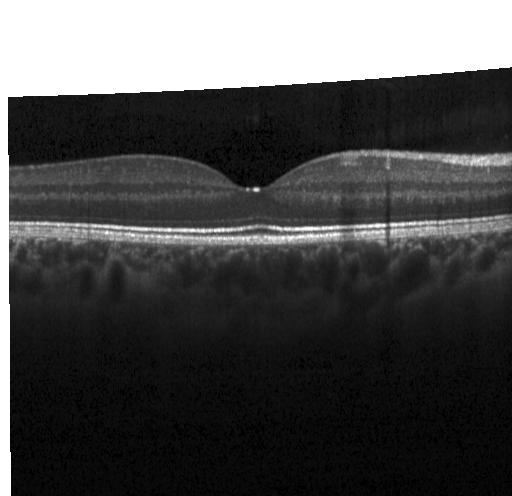

OCT B-scan — Neither CNV, DME, nor drusen.